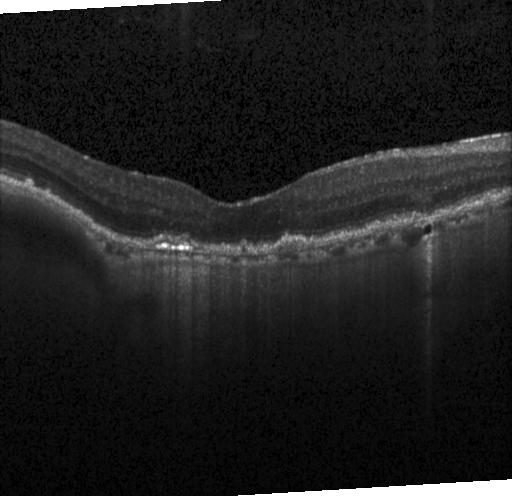
Fovea-centered; instrument: Heidelberg Spectralis; optical coherence tomography B-scan — Diagnosis: a choroidal neovascular membrane.